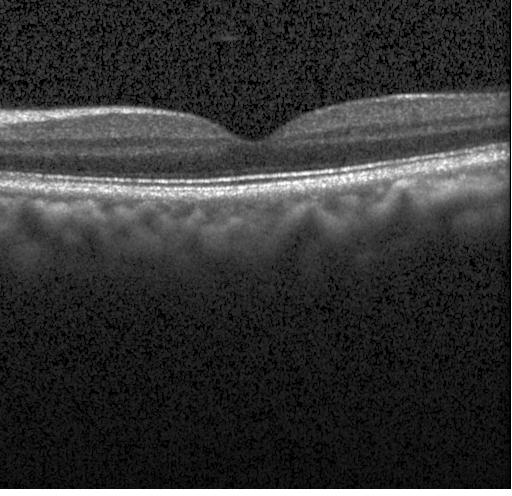
Heidelberg Spectralis OCT system, macular scan, SD-OCT, optical coherence tomography scan
Macular OCT: no choroidal neovascularization, no diabetic macular edema, and no drusen.